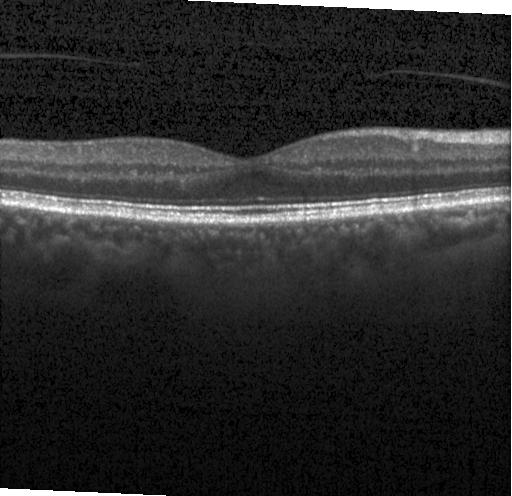
Macular OCT: no CNV, DME, or drusen.